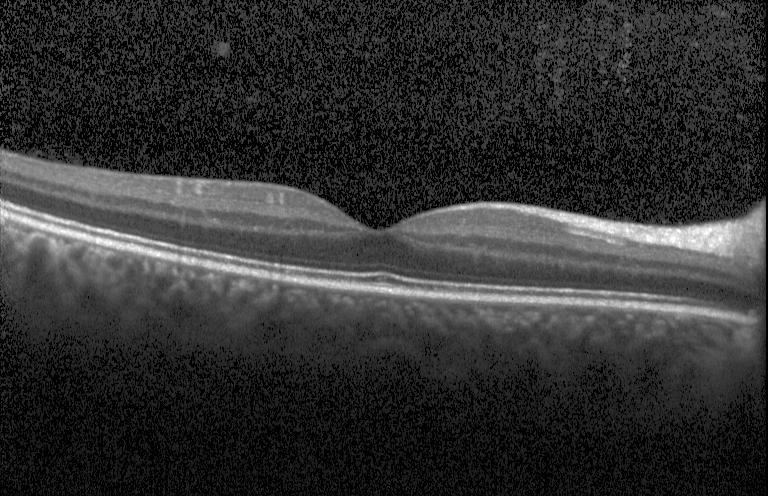
Diagnosis: no evidence of choroidal neovascularization, diabetic macular edema, or drusen.